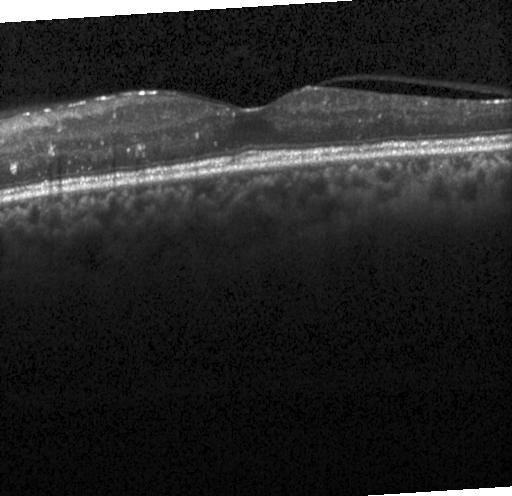
OCT line scan. Spectral-domain optical coherence tomography. Acquired on a Heidelberg Spectralis. Horizontal scan through the fovea — Dx: DME.